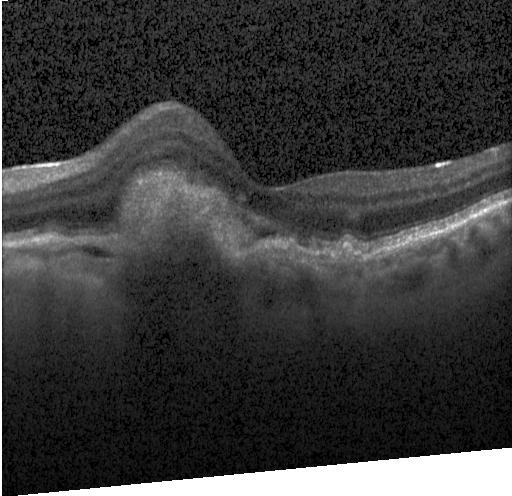 Finding: choroidal neovascularization.